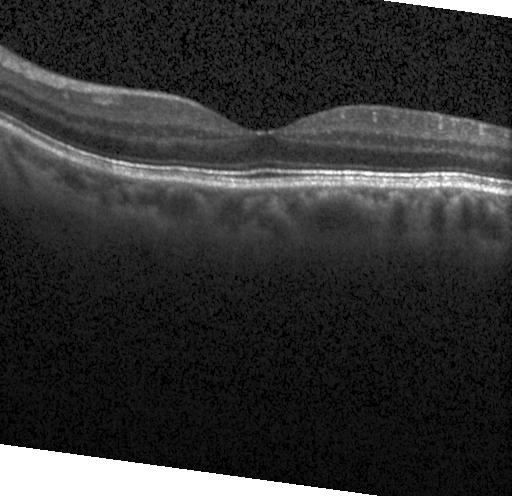
Optical coherence tomography B-scan — Macular OCT: no CNV, no DME, and no drusen.